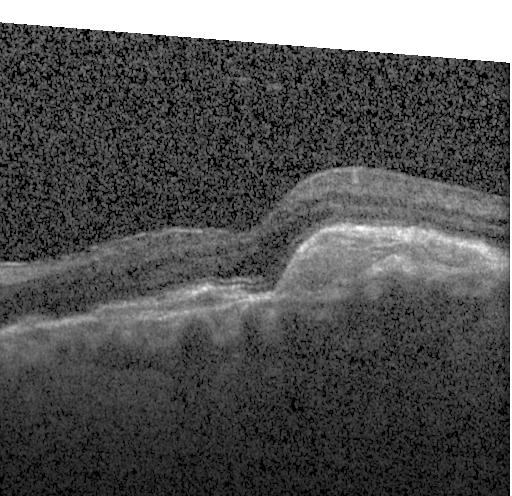

Retinal OCT cross-section. SD-OCT — Impression: a choroidal neovascular membrane.